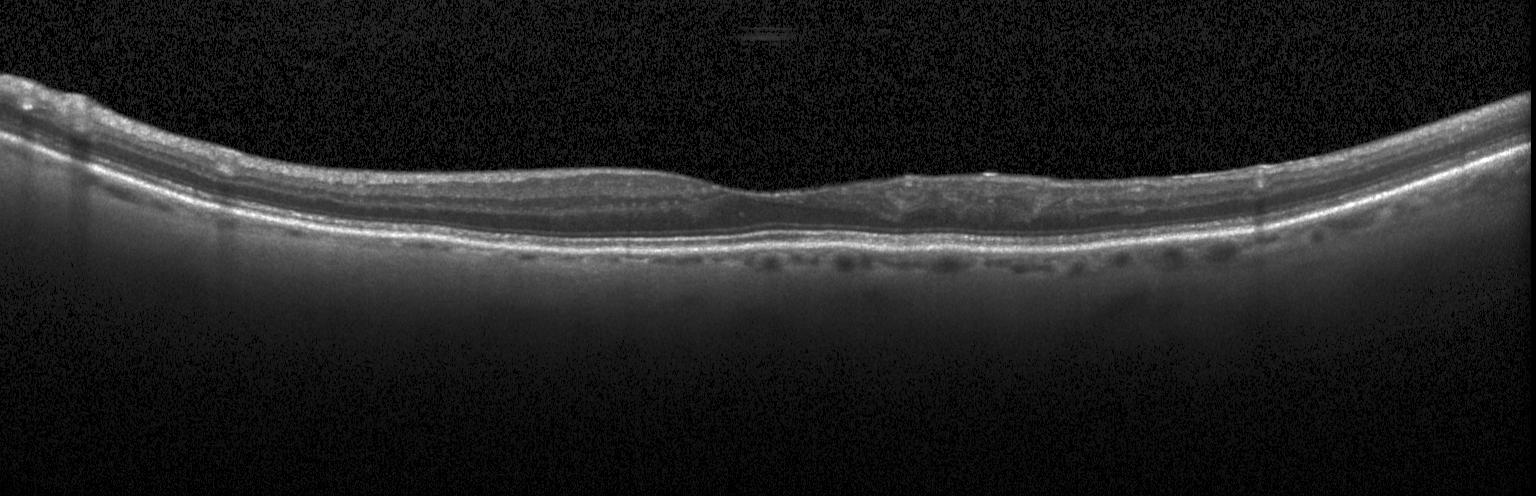 Retinal OCT cross-section, spectral-domain optical coherence tomography, centered on the fovea, instrument: Heidelberg Spectralis.
Diagnosis: no evidence of choroidal neovascularization, diabetic macular edema, or drusen.